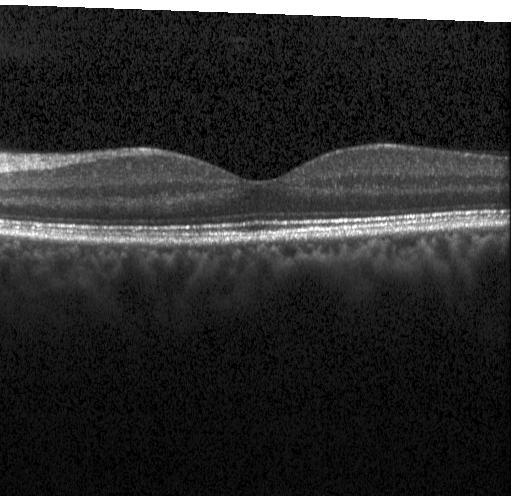 Instrument: Heidelberg Spectralis; optical coherence tomography scan.
Impression: no CNV, DME, or drusen.